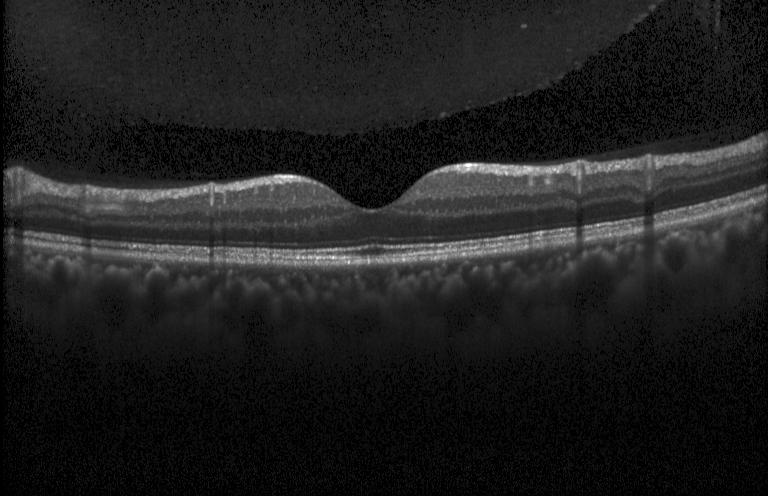 OCT B-scan
Impression: neither choroidal neovascularization, diabetic macular edema, nor drusen.